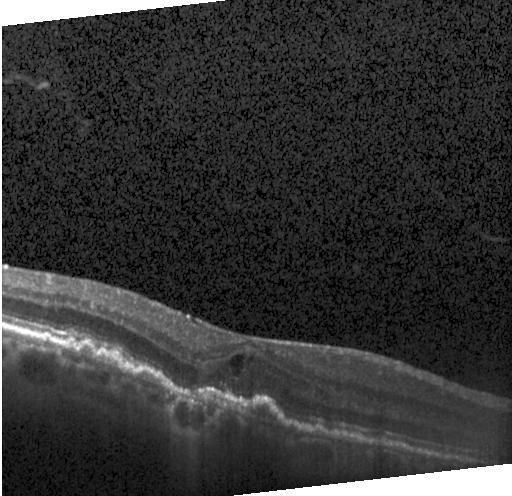
Retinal OCT cross-section · Heidelberg Spectralis · fovea-centered · SD-OCT — Impression: a choroidal neovascular membrane.